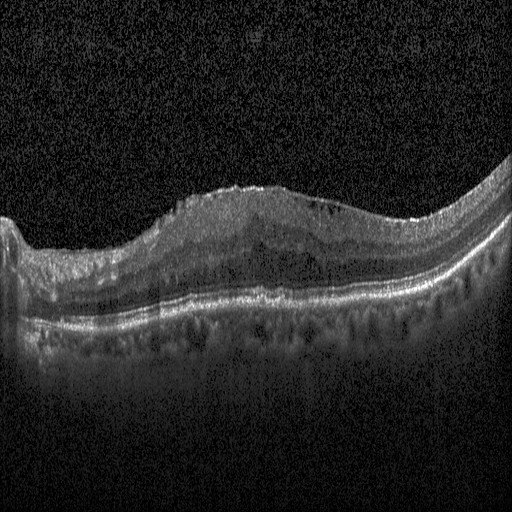 Diagnosis: DME.